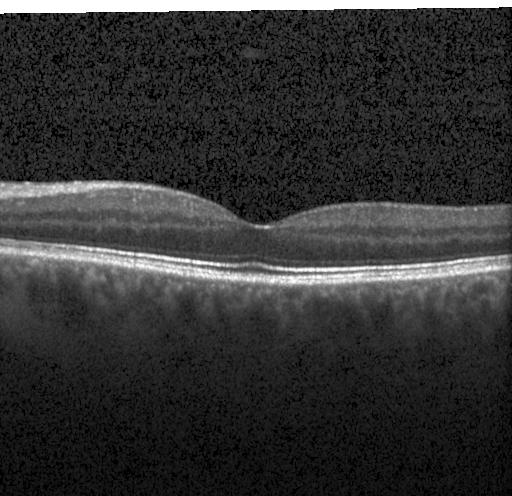
This B-scan demonstrates no evidence of CNV, DME, or drusen.